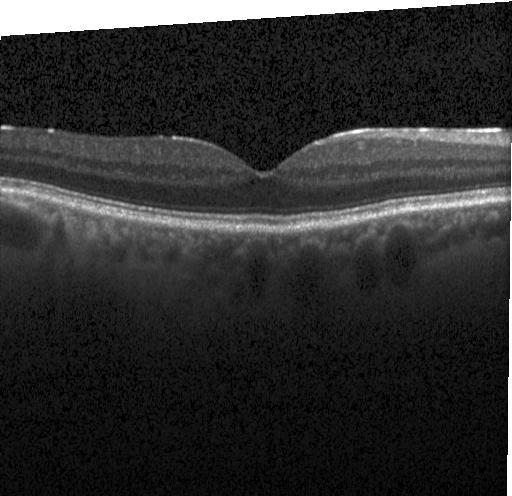 Impression: no CNV, DME, or drusen.